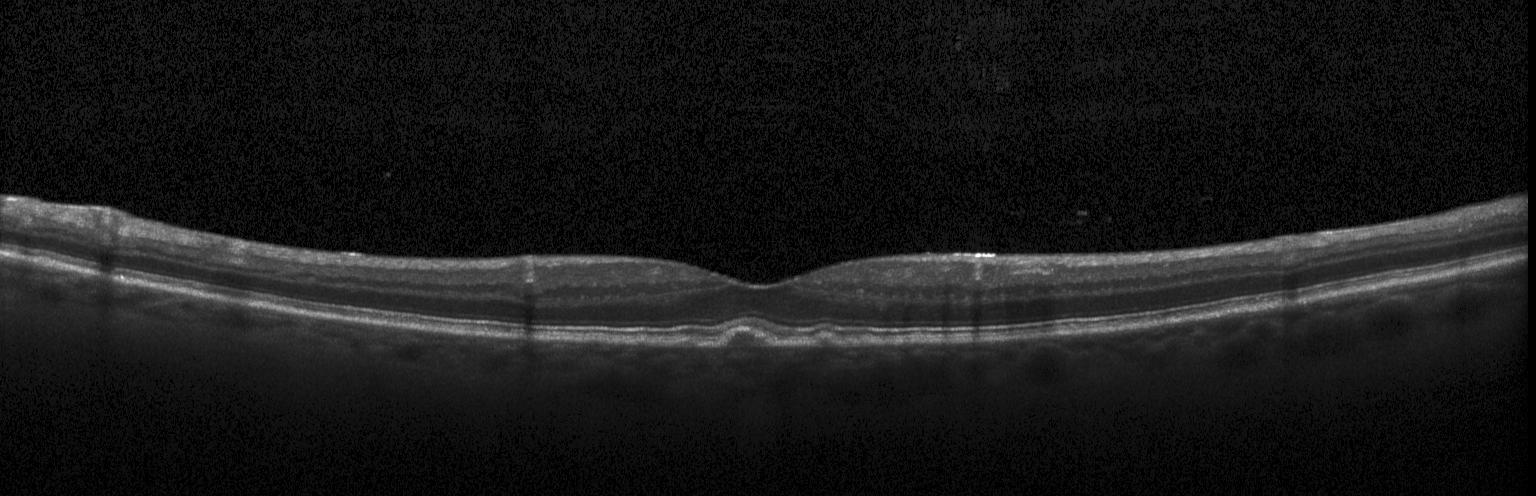 OCT B-scan; Heidelberg Spectralis
Assessment: sub-RPE drusenoid deposits.